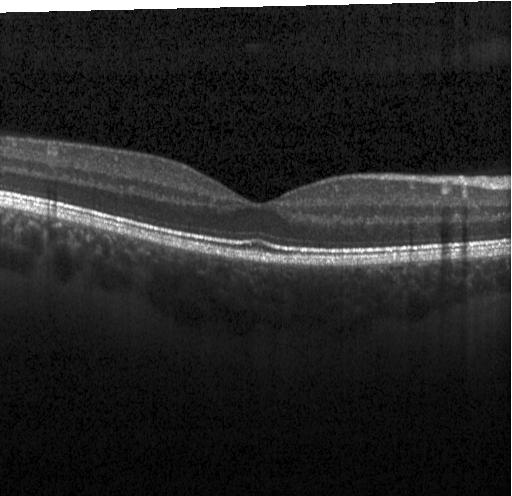
OCT line scan, acquired on a Heidelberg Spectralis, through the macula — Assessment: no choroidal neovascularization, diabetic macular edema, or drusen.